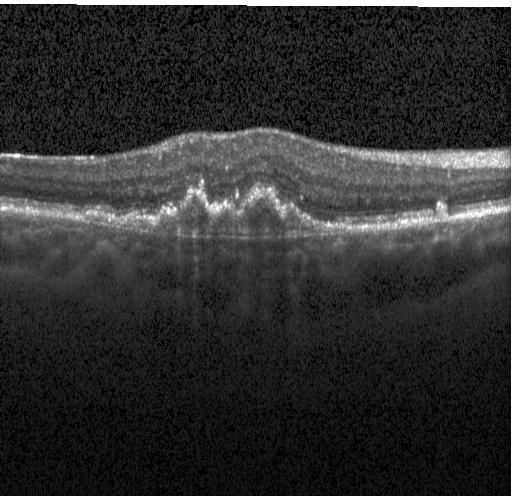
Instrument: Heidelberg Spectralis, OCT line scan.
The scan shows a choroidal neovascular membrane.